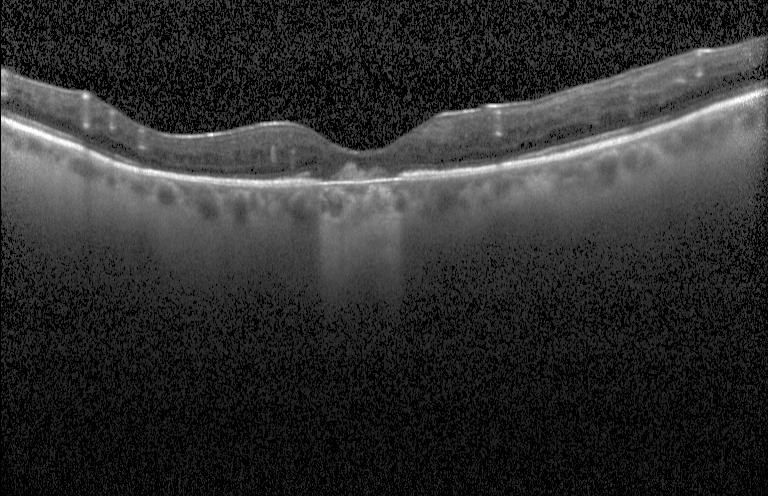
Macular OCT: a choroidal neovascular membrane.